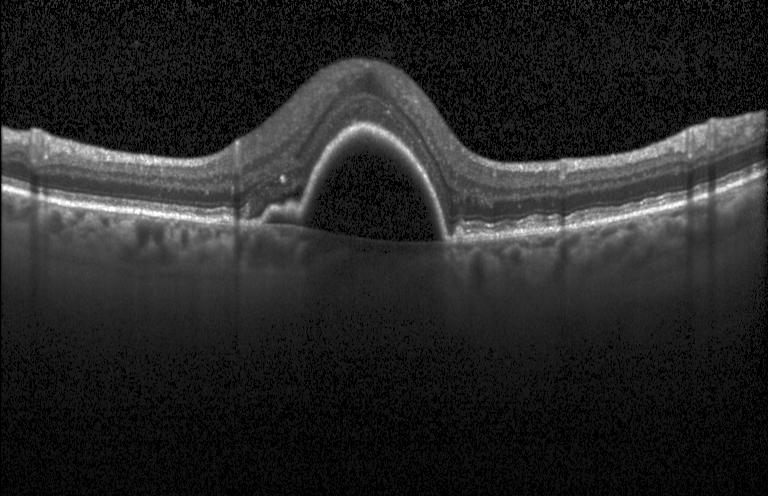
Spectral-domain OCT B-scan: a choroidal neovascular membrane.